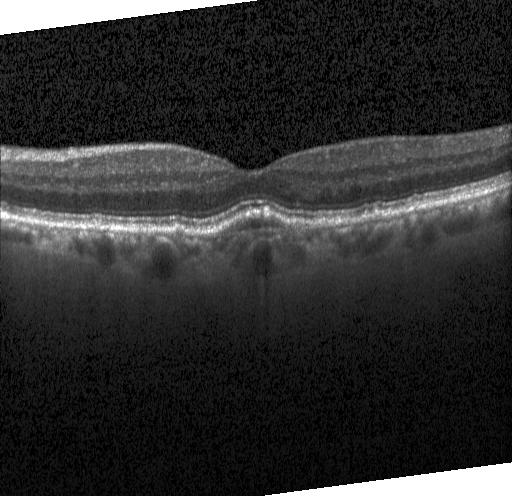
Spectral-domain OCT; OCT line scan; fovea-centered; Heidelberg Spectralis
This B-scan demonstrates a choroidal neovascular membrane.